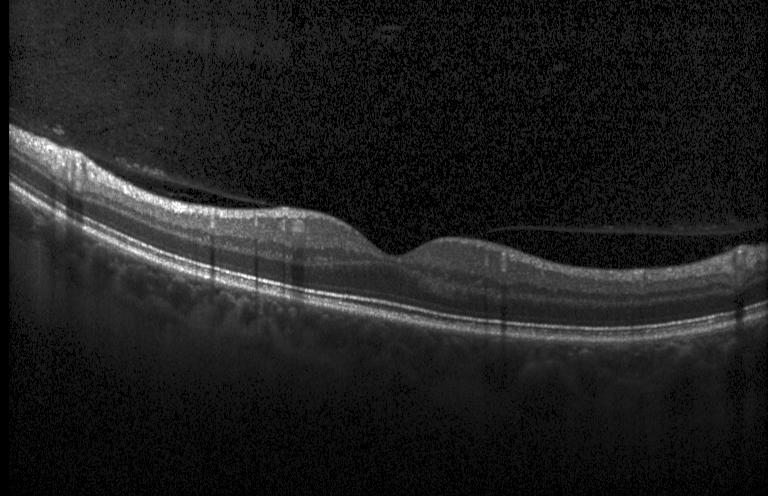

Optical coherence tomography B-scan; SD-OCT
Dx: no choroidal neovascularization, no diabetic macular edema, and no drusen.